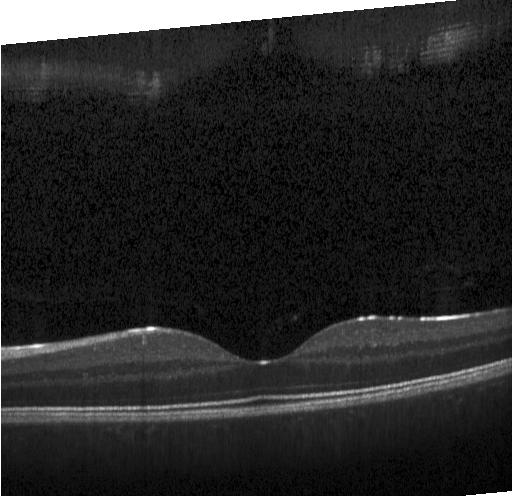
Diagnosis: neither CNV, DME, nor drusen.